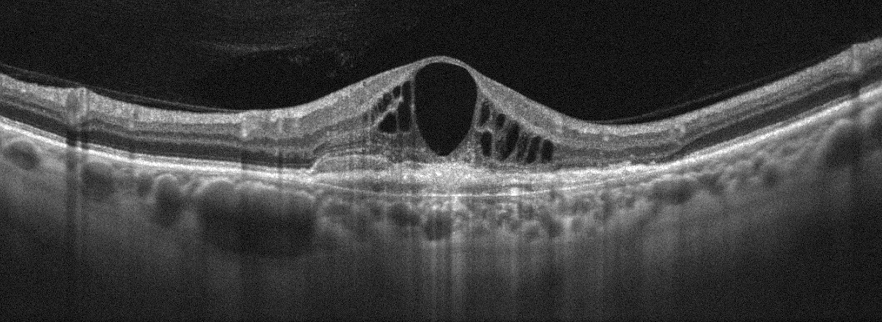

Optical coherence tomography B-scan · through the macula · oculus sinister — OCT finding: age-related macular degeneration (AMD).